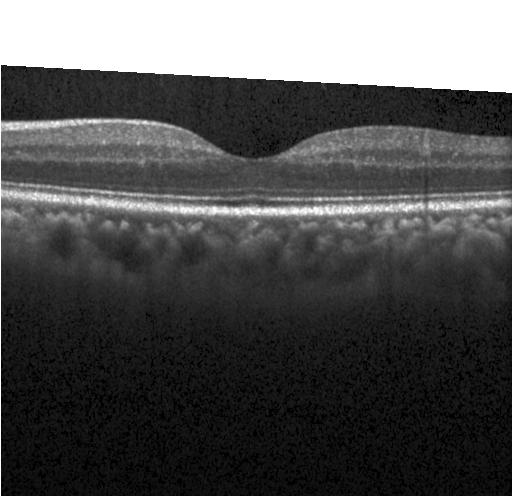

OCT finding: neither CNV, DME, nor drusen.